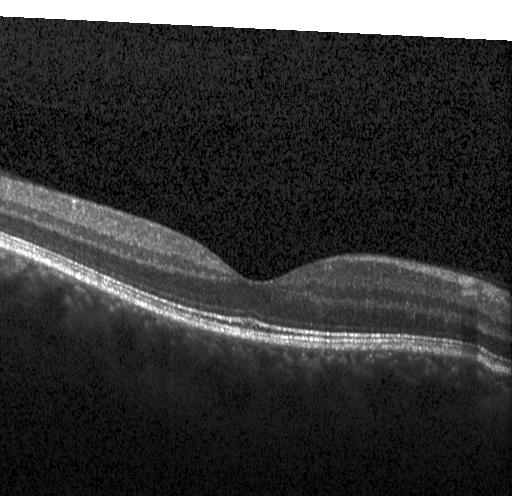

This B-scan demonstrates no choroidal neovascularization, diabetic macular edema, or drusen.